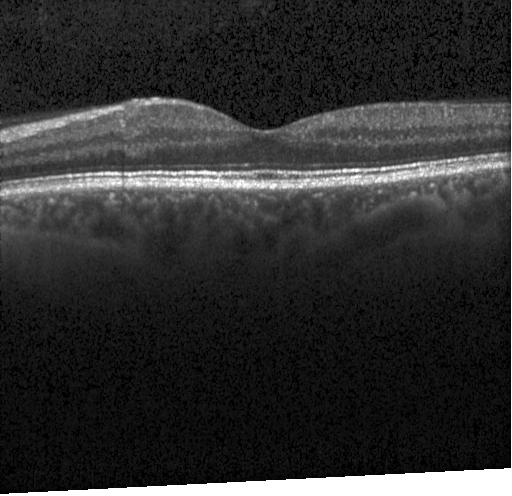
OCT scan showing no CNV, no DME, and no drusen.